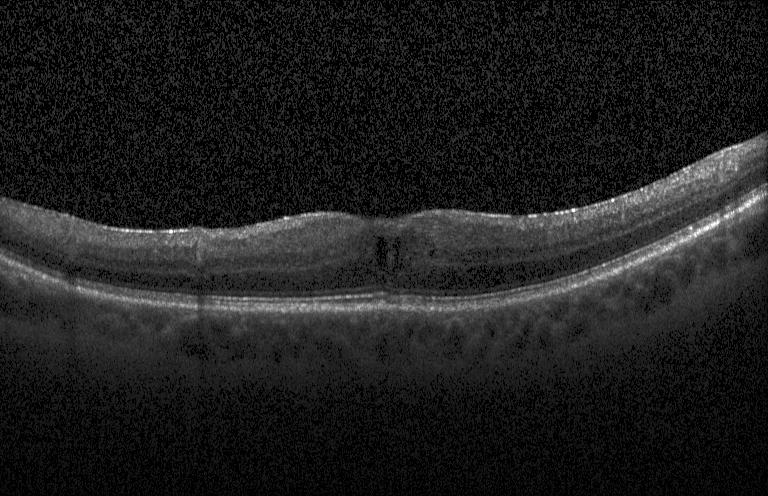

OCT line scan.
This B-scan demonstrates DME.